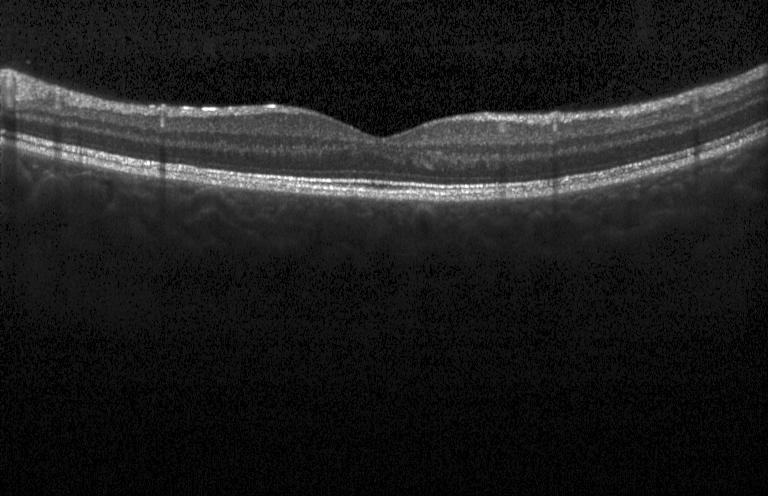 Optical coherence tomography scan; instrument: Heidelberg Spectralis.
Macular OCT: no evidence of choroidal neovascularization, diabetic macular edema, or drusen.